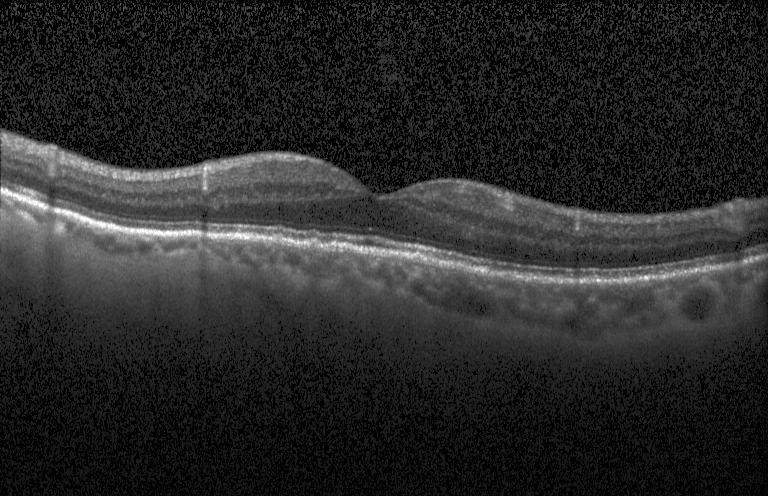
Assessment: no evidence of choroidal neovascularization, diabetic macular edema, or drusen.